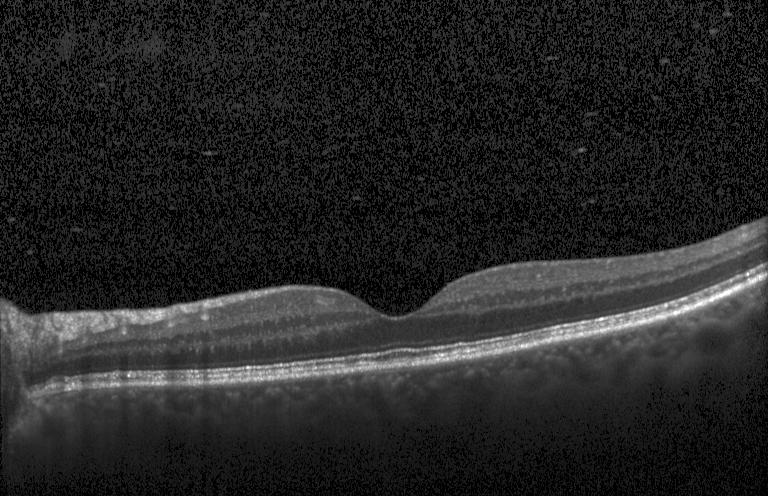 Spectral-domain optical coherence tomography; instrument: Heidelberg Spectralis; centered on the fovea; optical coherence tomography B-scan. The scan shows no CNV, DME, or drusen.